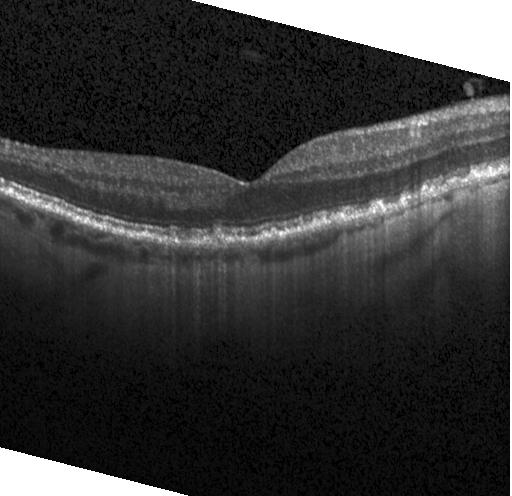

Optical coherence tomography scan.
Dx: multiple drusen.